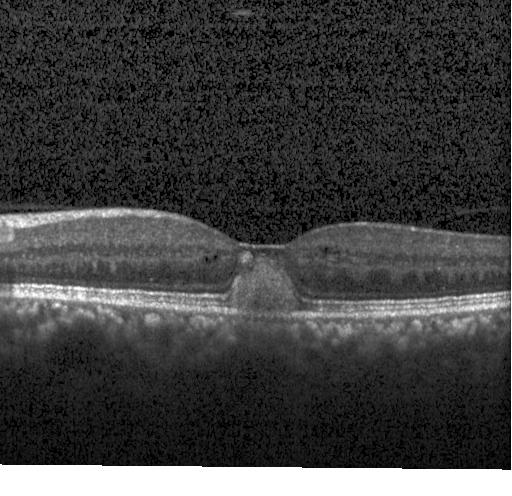
Dx: a choroidal neovascular membrane.